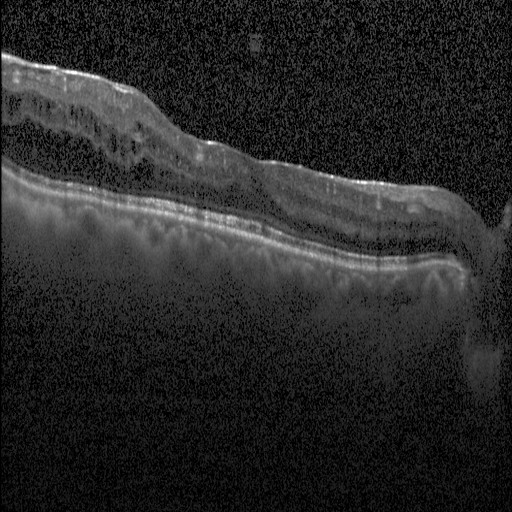

Heidelberg Spectralis OCT system; horizontal scan through the fovea; optical coherence tomography scan; spectral-domain optical coherence tomography. Diabetic macular edema.